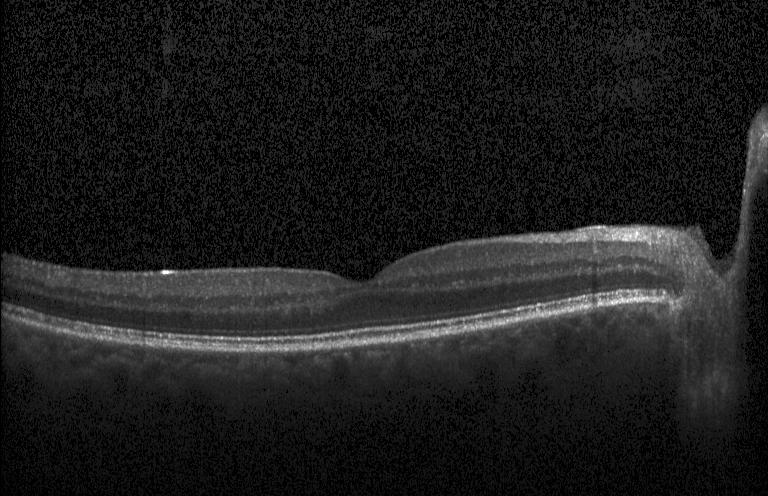 Horizontal scan through the fovea, OCT line scan.
Impression: neither choroidal neovascularization, diabetic macular edema, nor drusen.